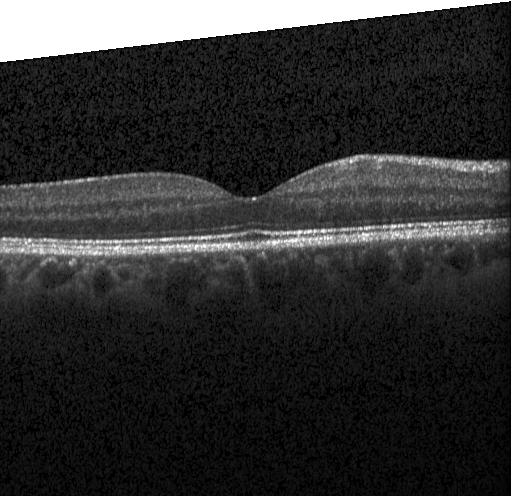

OCT scan showing neither choroidal neovascularization, diabetic macular edema, nor drusen.